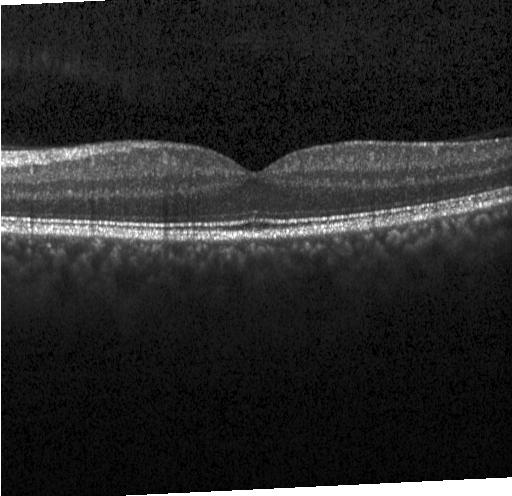

Diagnosis: no choroidal neovascularization, diabetic macular edema, or drusen.